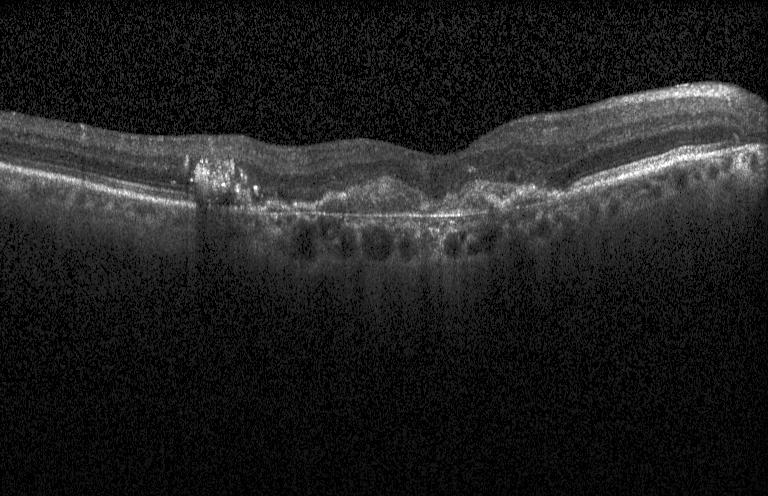
Dx: CNV.